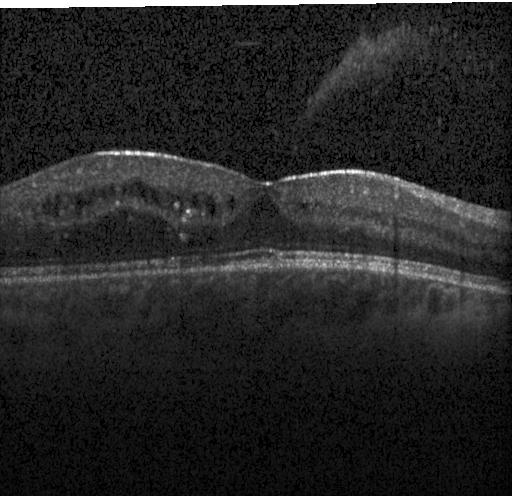

OCT line scan. Dx: DME.